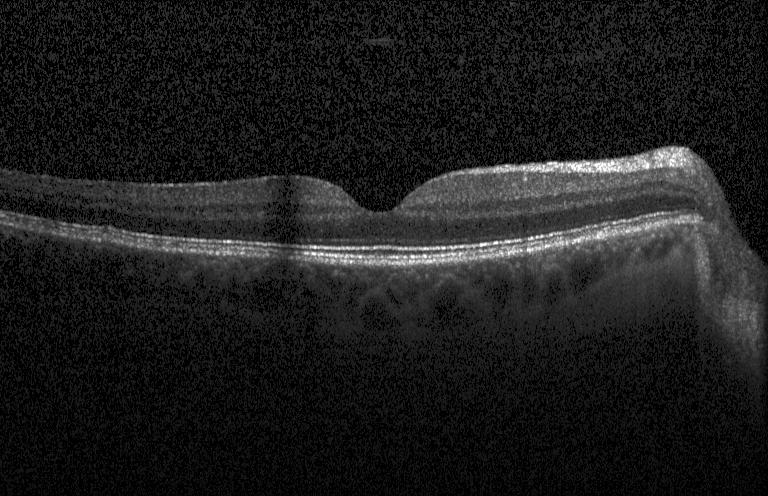

Retinal OCT B-scan — Dx: neither CNV, DME, nor drusen.